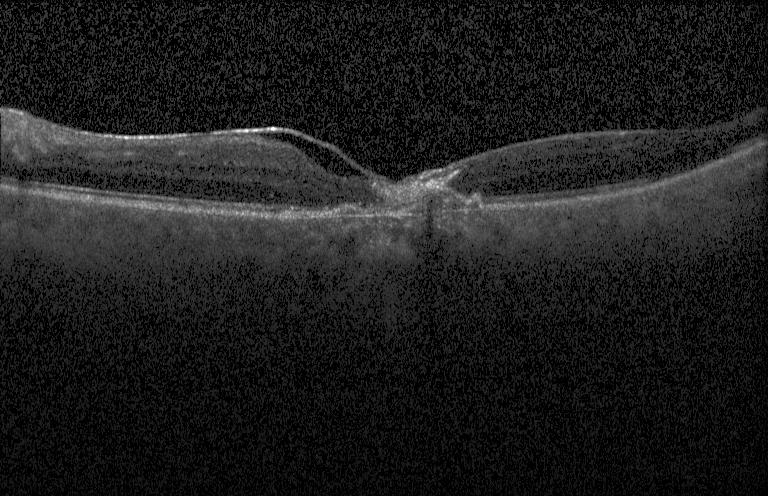 Finding: a choroidal neovascular membrane.